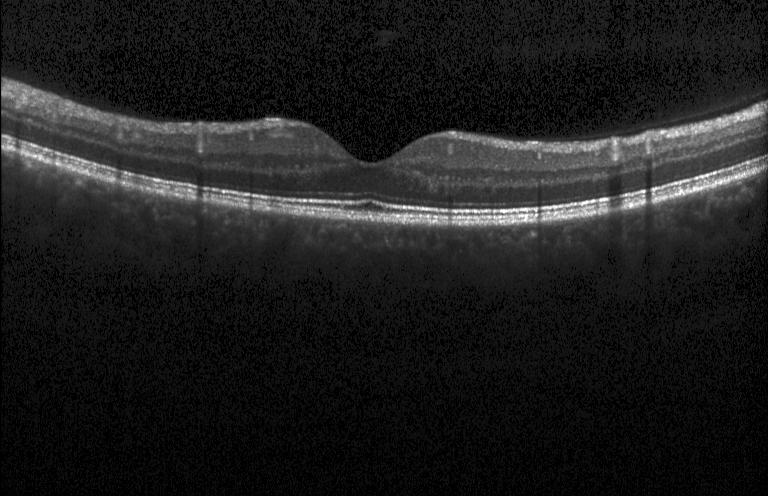
Retinal OCT cross-section · acquired on a Heidelberg Spectralis · SD-OCT. No choroidal neovascularization, diabetic macular edema, or drusen.